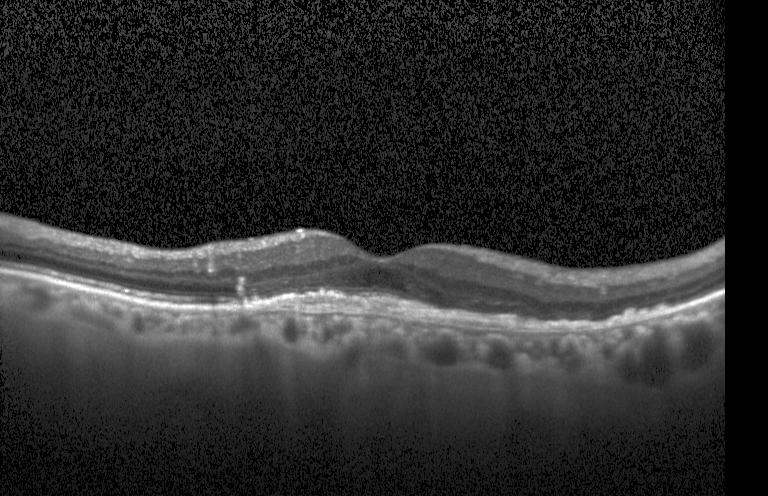
OCT B-scan. Finding: CNV.